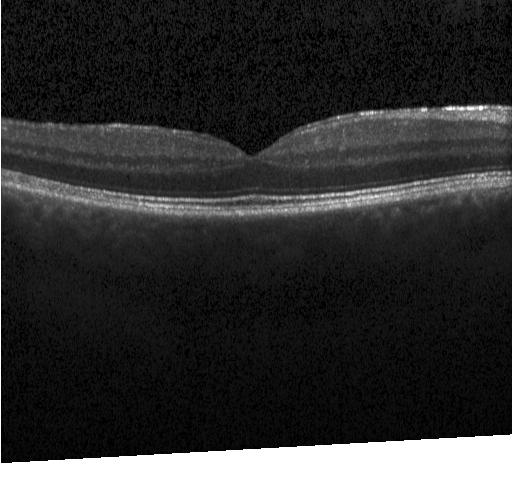

Diagnosis: no CNV, DME, or drusen.